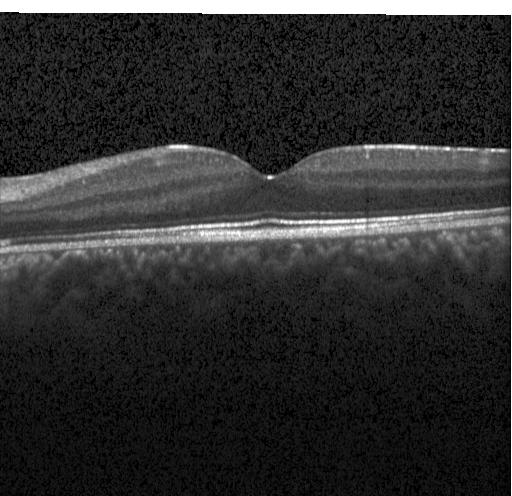
Heidelberg Spectralis OCT system · optical coherence tomography B-scan
OCT finding: neither choroidal neovascularization, diabetic macular edema, nor drusen.